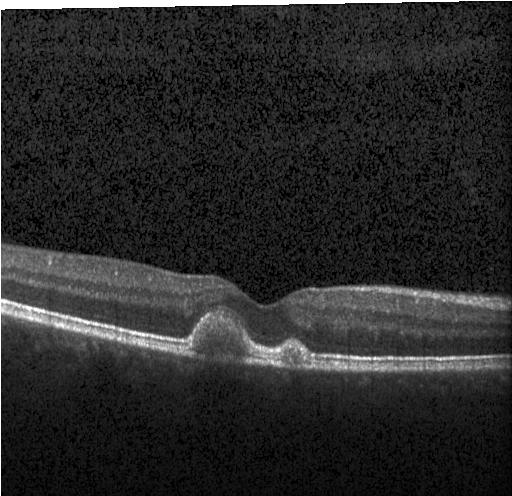 OCT scan showing sub-RPE drusenoid deposits.